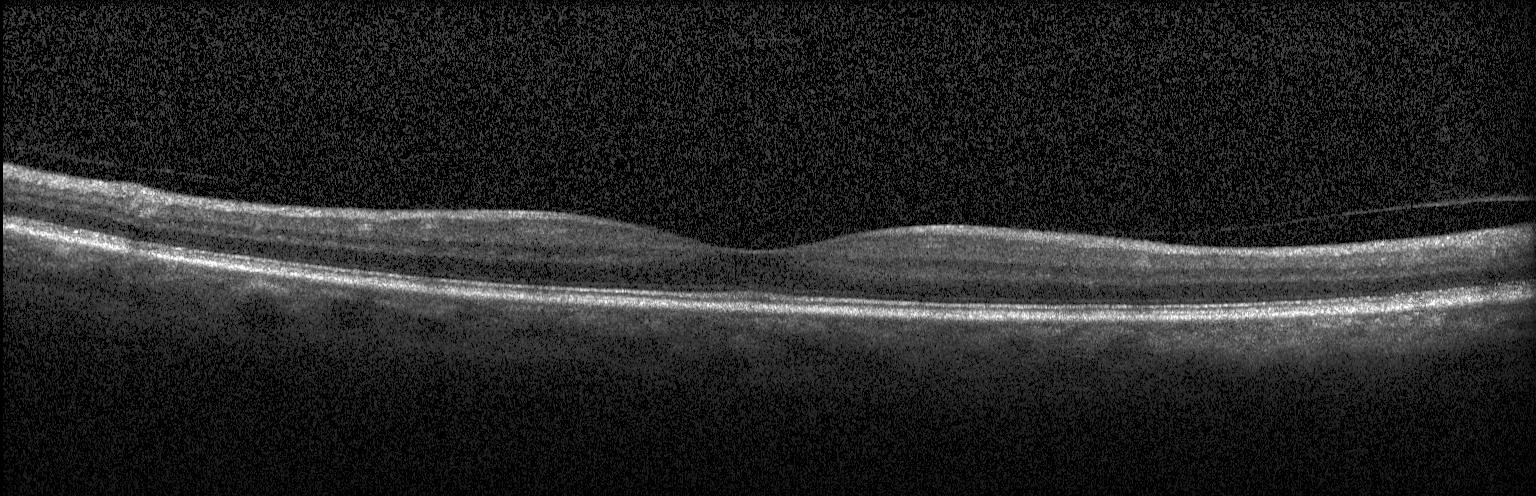

Diagnosis: no choroidal neovascularization, no diabetic macular edema, and no drusen.